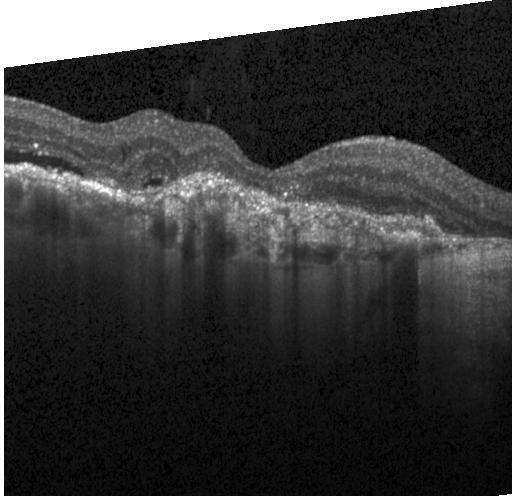

Instrument: Heidelberg Spectralis · spectral-domain optical coherence tomography · retinal OCT B-scan — This B-scan demonstrates choroidal neovascularization.